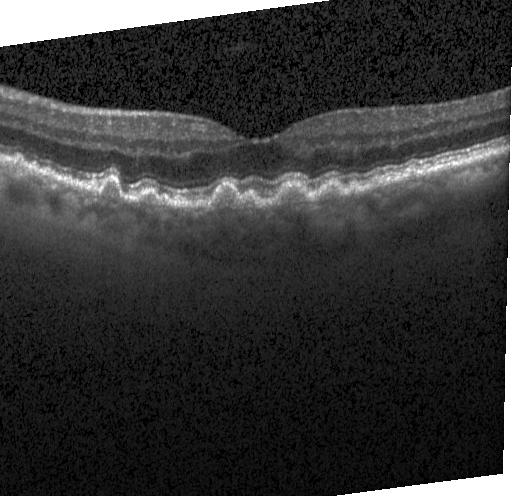 Diagnosis: sub-RPE drusenoid deposits.